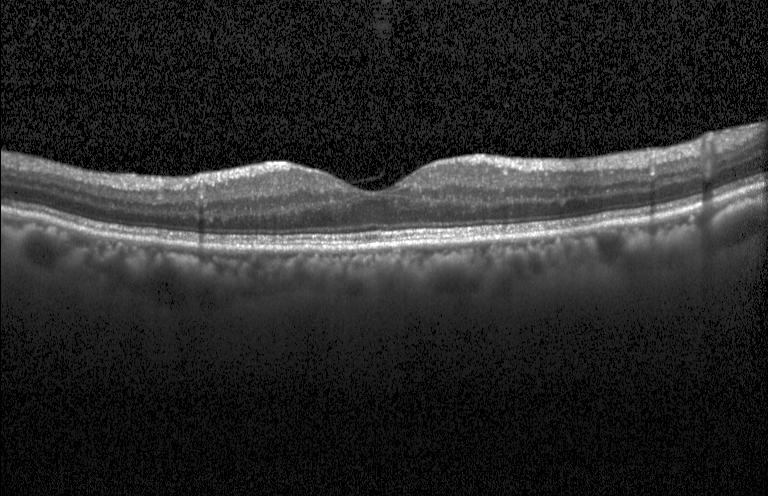

Retinal OCT B-scan. OCT finding: no choroidal neovascularization, diabetic macular edema, or drusen.